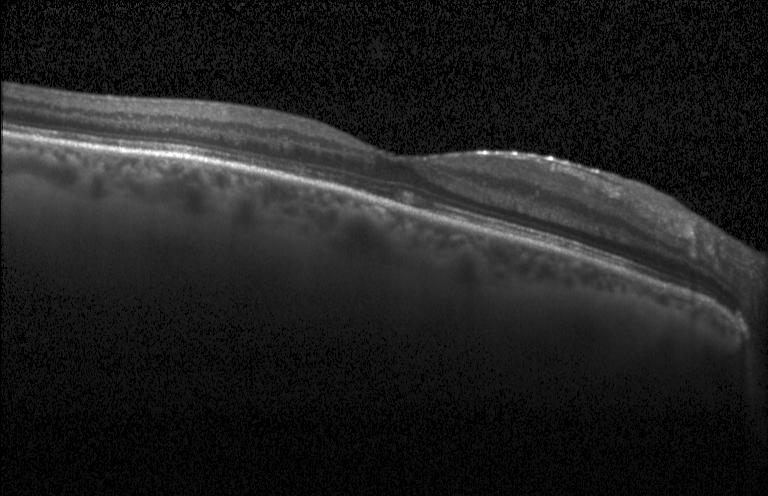 OCT line scan. No CNV, DME, or drusen.